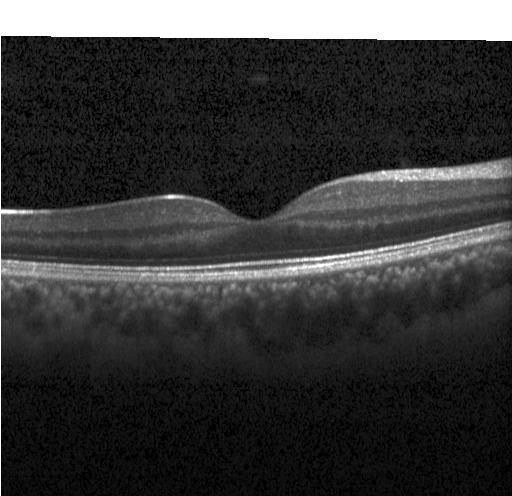
OCT B-scan. Acquired on a Heidelberg Spectralis. Diagnosis: no choroidal neovascularization, no diabetic macular edema, and no drusen.